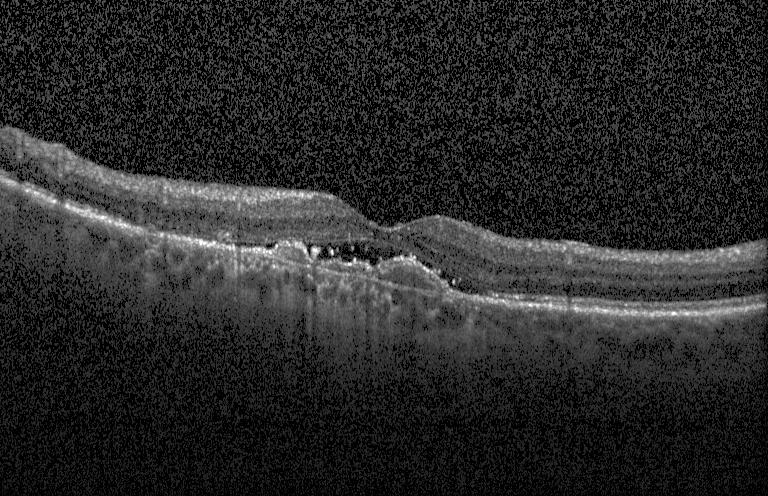
Centered on the fovea · retinal OCT B-scan · Heidelberg Spectralis. Finding: a choroidal neovascular membrane.